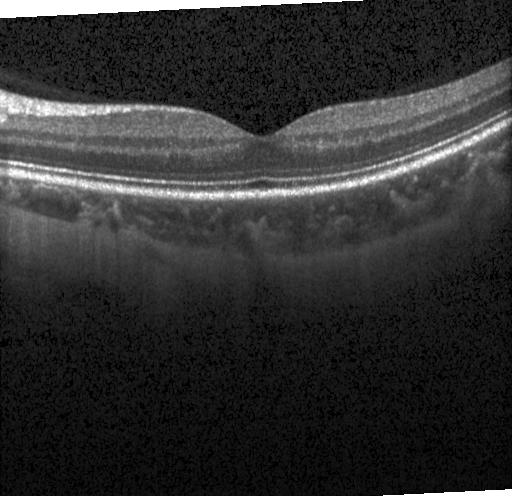
Impression: no evidence of choroidal neovascularization, diabetic macular edema, or drusen.